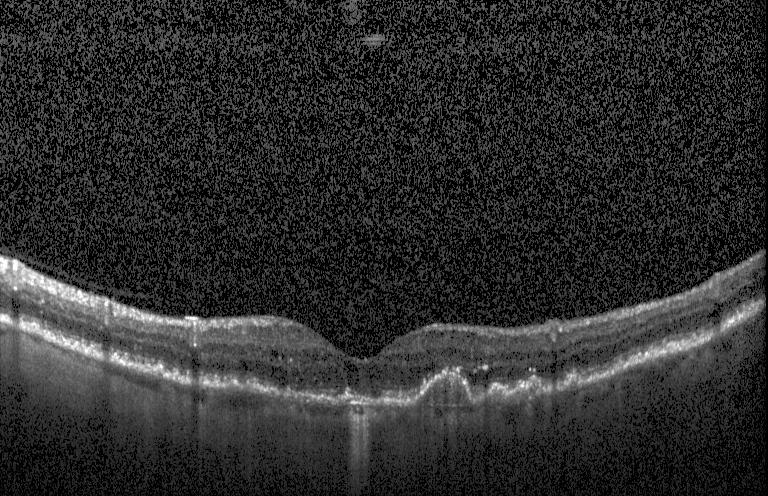

Impression: CNV.